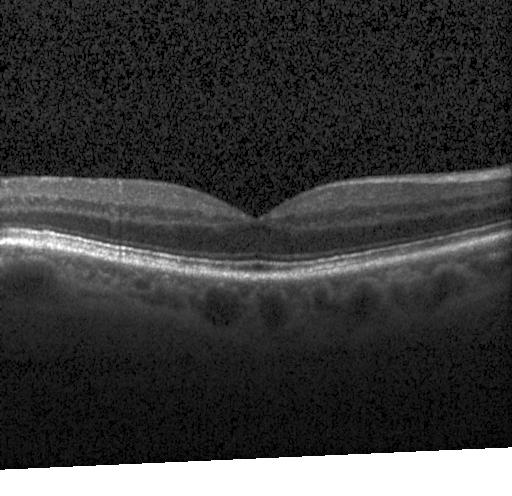

Retinal OCT cross-section showing neither choroidal neovascularization, diabetic macular edema, nor drusen.